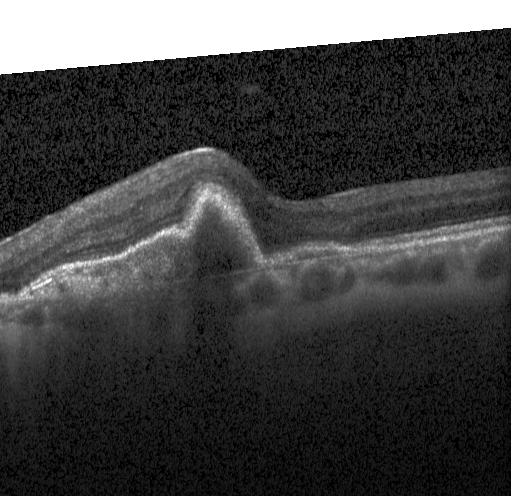

CNV.